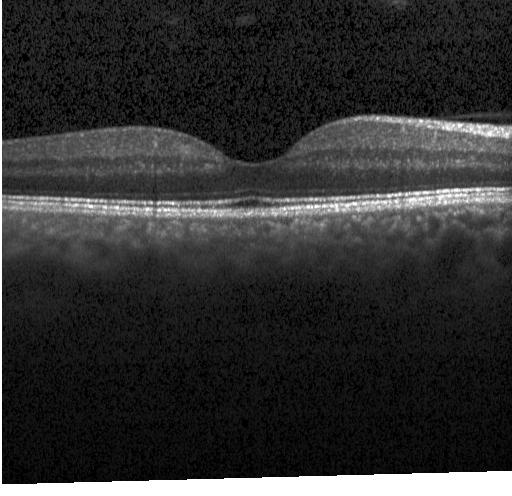
Spectral-domain optical coherence tomography · centered on the fovea · acquired on a Heidelberg Spectralis · optical coherence tomography scan. Assessment: no choroidal neovascularization, diabetic macular edema, or drusen.